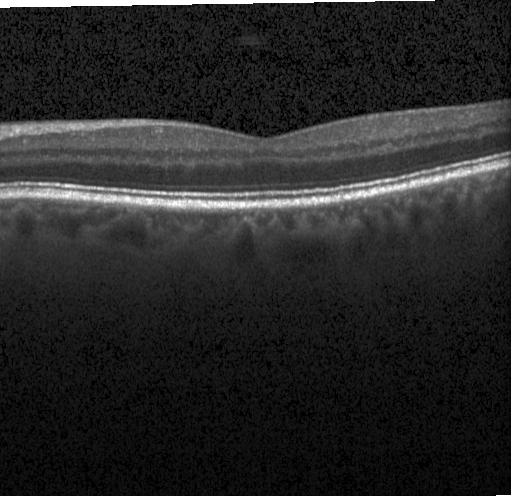 Spectral-domain OCT. Optical coherence tomography scan. Through the macula. Instrument: Heidelberg Spectralis — Finding: no CNV, DME, or drusen.